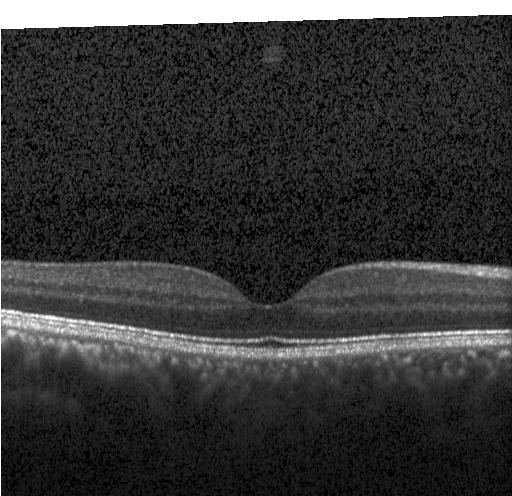
Instrument: Heidelberg Spectralis; retinal OCT B-scan — This B-scan demonstrates no evidence of choroidal neovascularization, diabetic macular edema, or drusen.